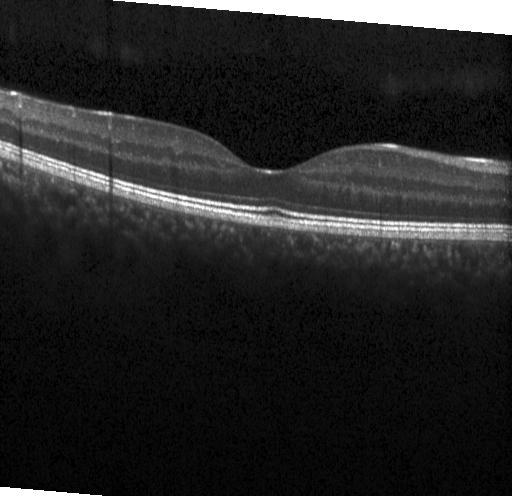 The scan shows neither choroidal neovascularization, diabetic macular edema, nor drusen.